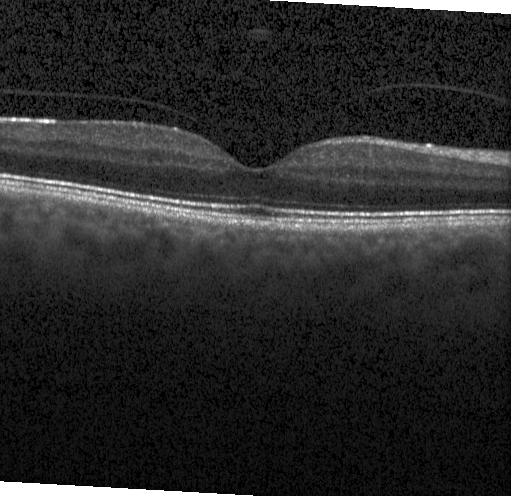 OCT B-scan. Through the macula.
Diagnosis: no evidence of choroidal neovascularization, diabetic macular edema, or drusen.